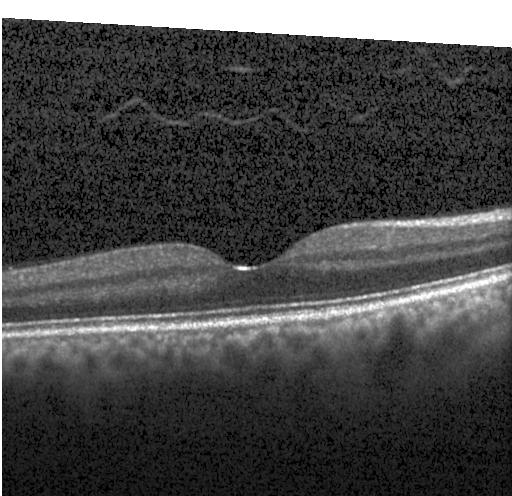 OCT B-scan — This B-scan demonstrates neither choroidal neovascularization, diabetic macular edema, nor drusen.